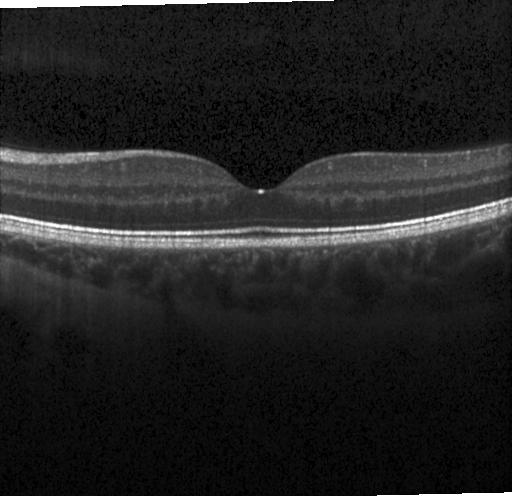
Finding: no choroidal neovascularization, diabetic macular edema, or drusen.